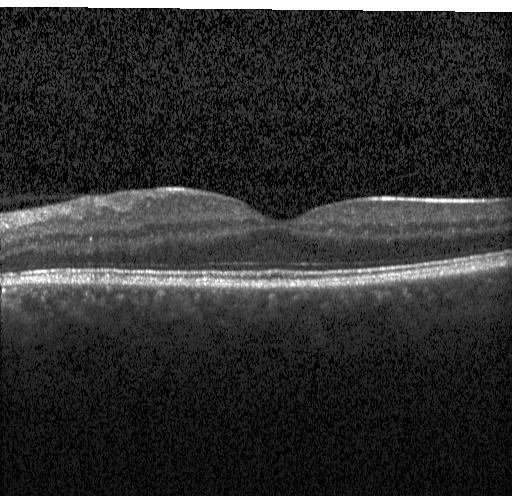

Assessment: neither CNV, DME, nor drusen.